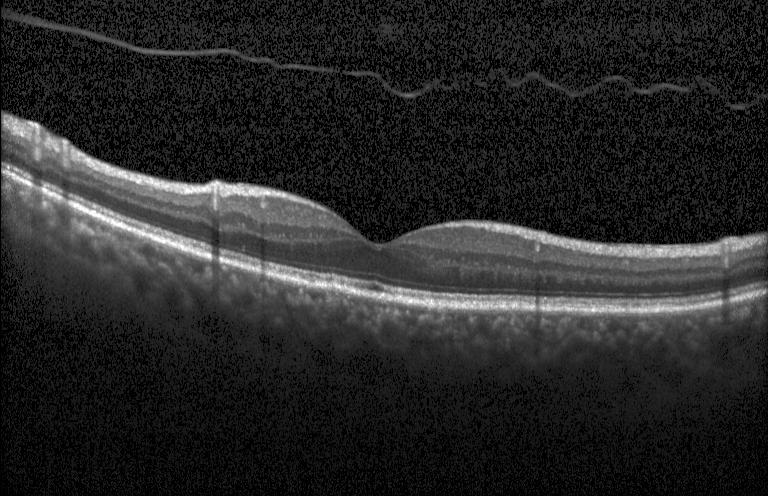

Macular scan, spectral-domain OCT, instrument: Heidelberg Spectralis, optical coherence tomography B-scan — Assessment: no CNV, no DME, and no drusen.